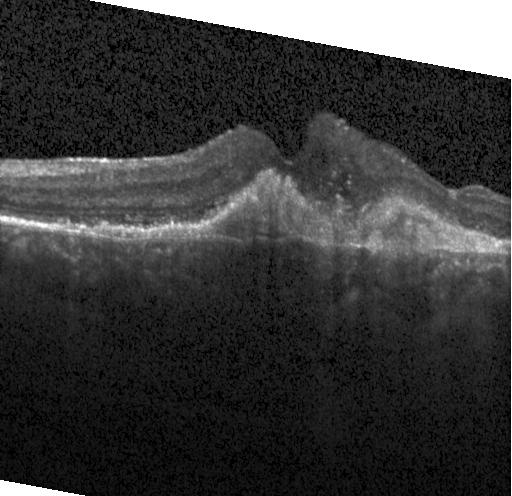
OCT B-scan.
The scan shows a choroidal neovascular membrane.